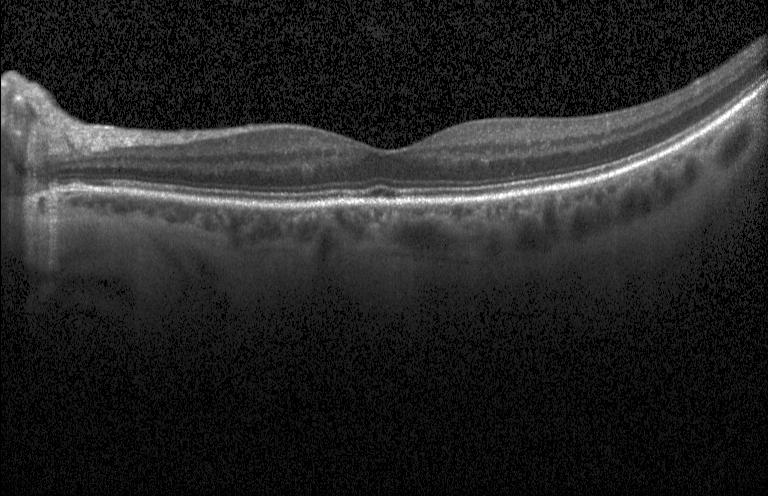 OCT B-scan — Finding: no evidence of choroidal neovascularization, diabetic macular edema, or drusen.